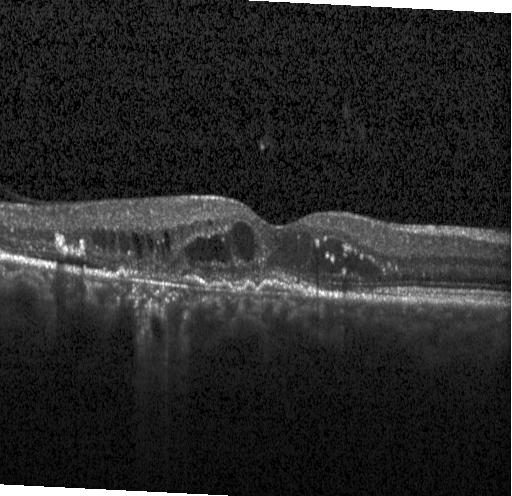
This B-scan demonstrates a choroidal neovascular membrane.